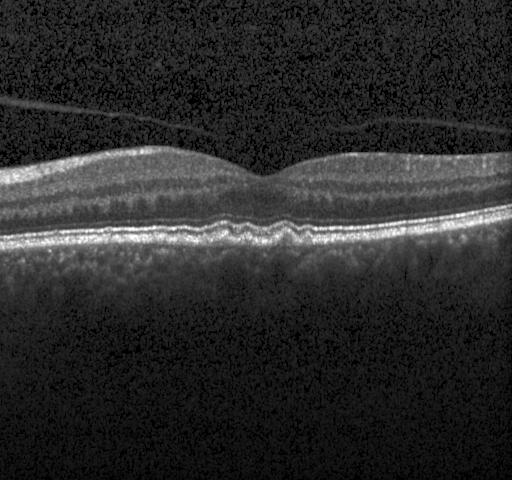

Horizontal scan through the fovea · retinal OCT cross-section — Macular OCT: sub-RPE drusenoid deposits.